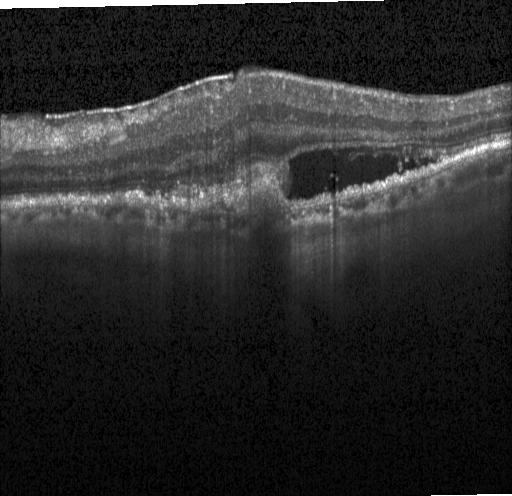 Impression: a choroidal neovascular membrane.